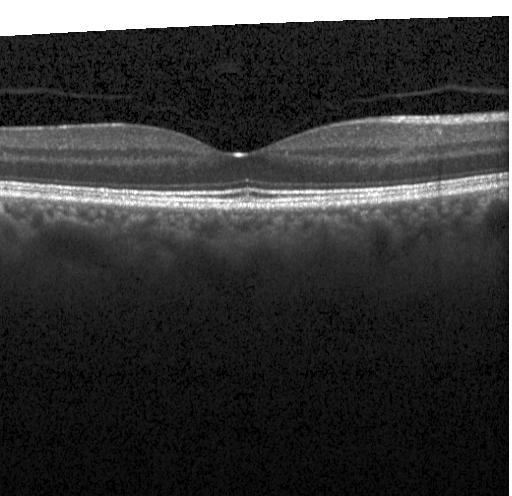 Spectral-domain OCT. OCT B-scan. No evidence of choroidal neovascularization, diabetic macular edema, or drusen.